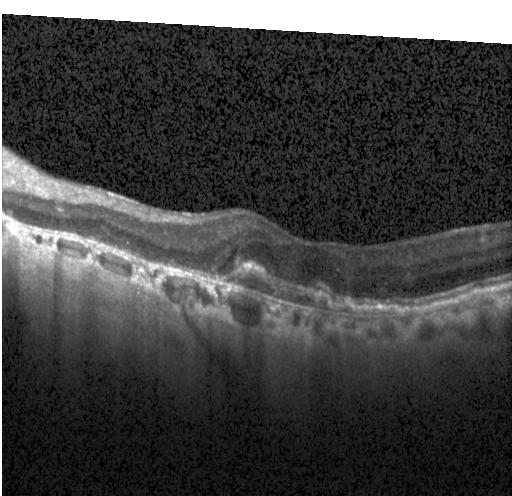
Retinal OCT cross-section showing a choroidal neovascular membrane.